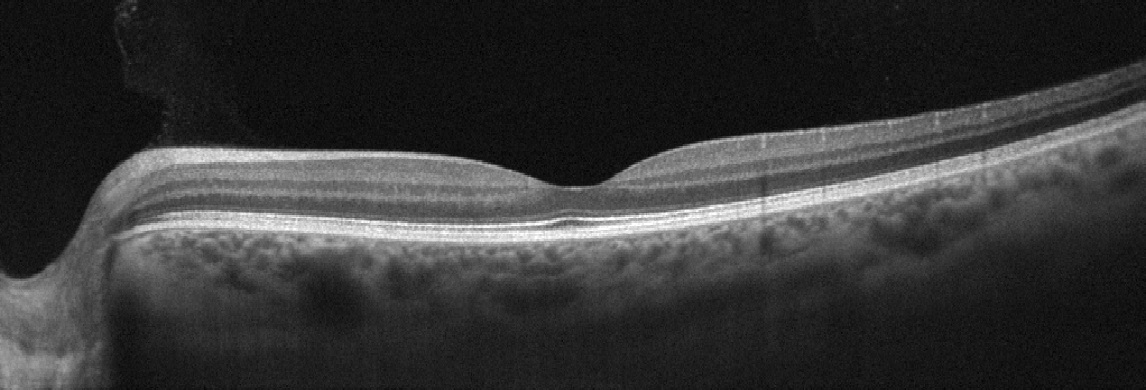

Optical coherence tomography scan, instrument: Optovue Avanti RTVue XR, macular scan.
No AMD, DME, ERM, RAO, RVO, or VID.